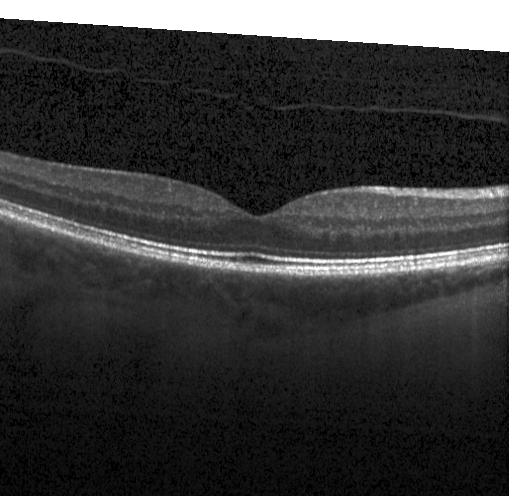
Optical coherence tomography scan
The scan shows no evidence of choroidal neovascularization, diabetic macular edema, or drusen.